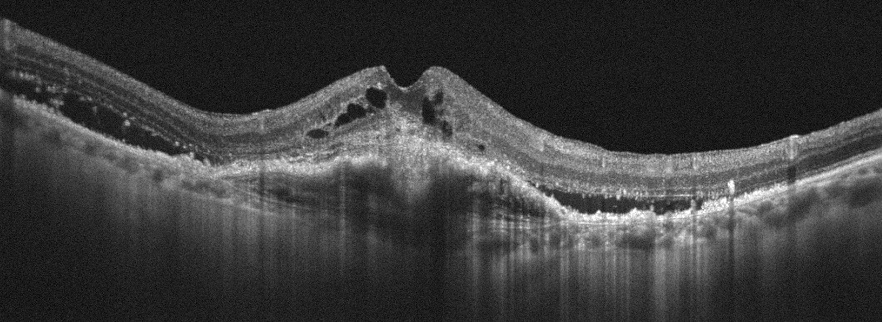
Optical coherence tomography scan — OCT finding: age-related macular degeneration (AMD).